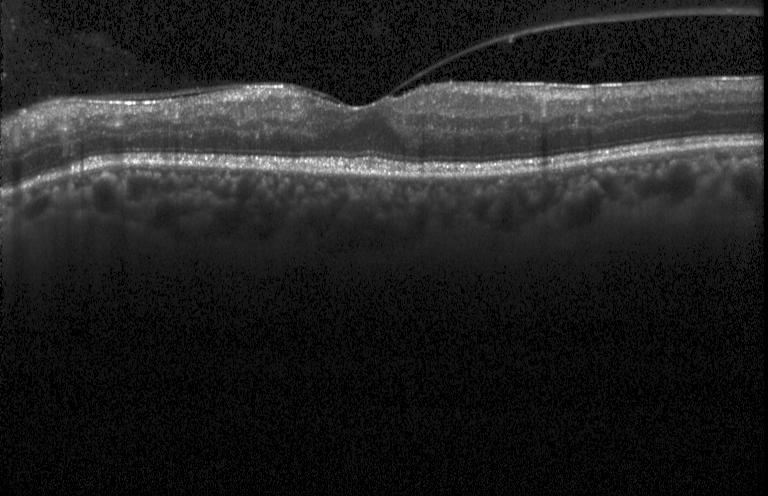 OCT B-scan showing diabetic macular edema.